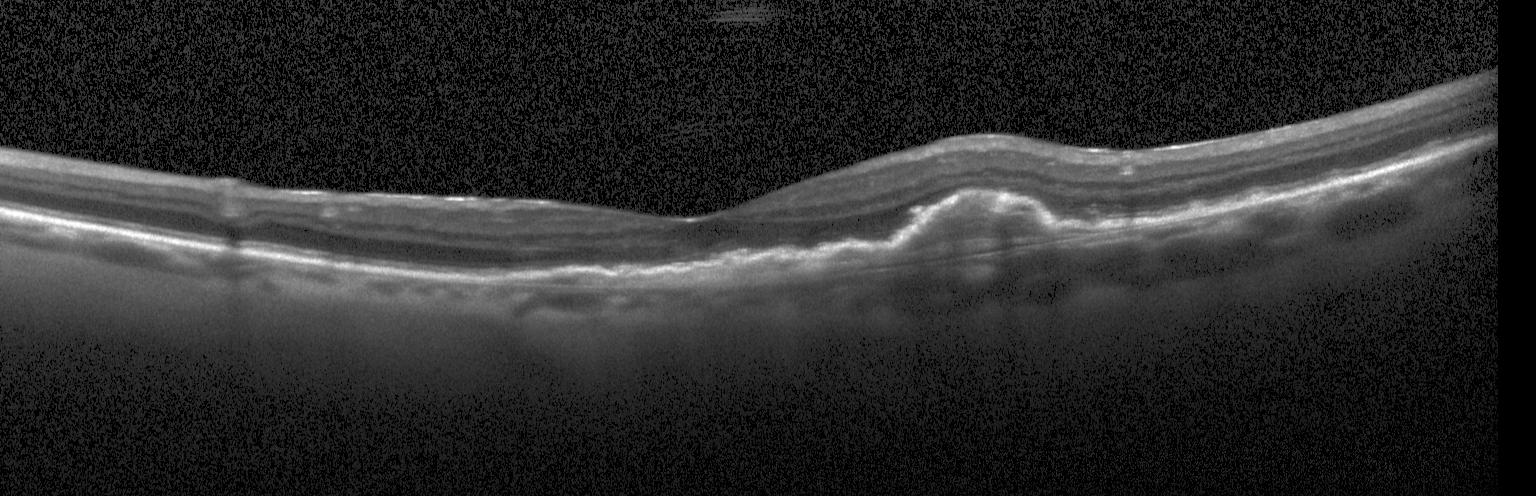

Impression: sub-RPE drusenoid deposits.